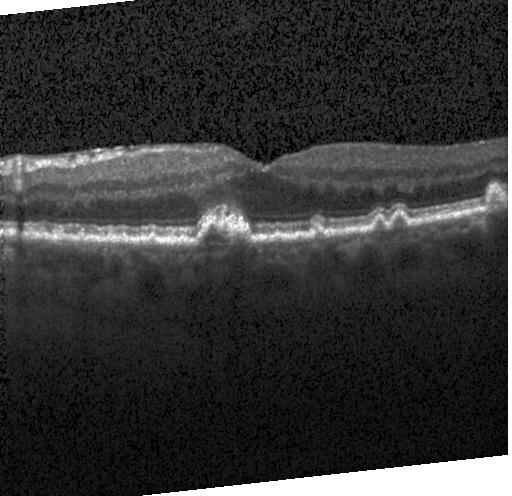

Acquired on a Heidelberg Spectralis. Horizontal scan through the fovea. Spectral-domain OCT. OCT B-scan — Multiple drusen.